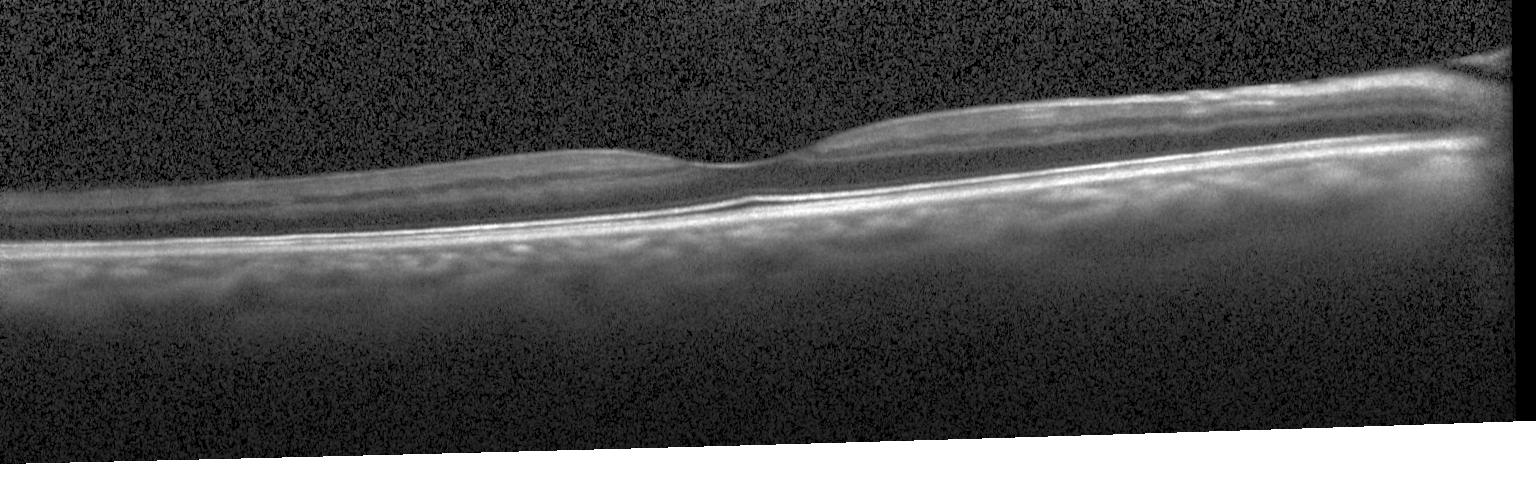
Dx: neither choroidal neovascularization, diabetic macular edema, nor drusen.